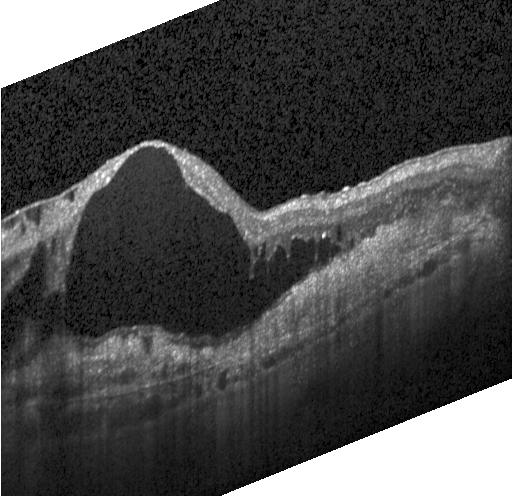

Optical coherence tomography scan · spectral-domain optical coherence tomography · acquired on a Heidelberg Spectralis
The scan shows a choroidal neovascular membrane.